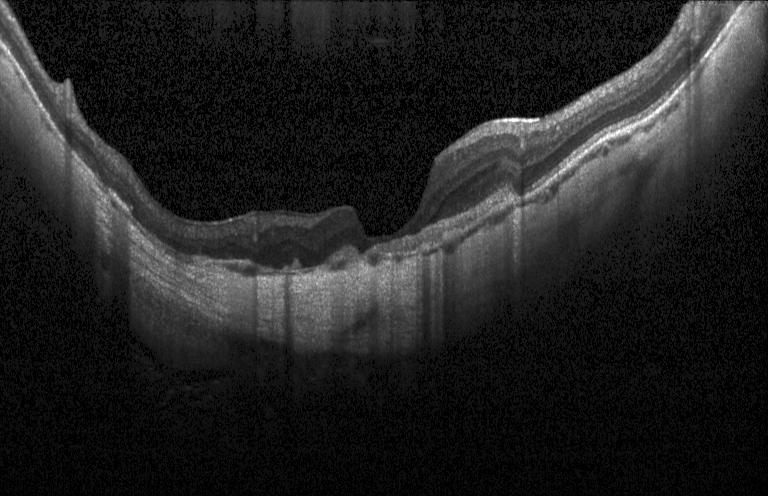 Impression: choroidal neovascularization (CNV).